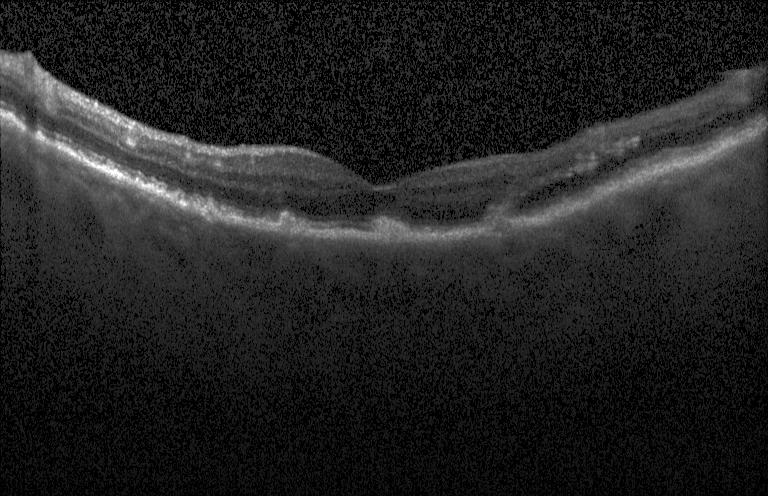
OCT line scan
Diagnosis: CNV.